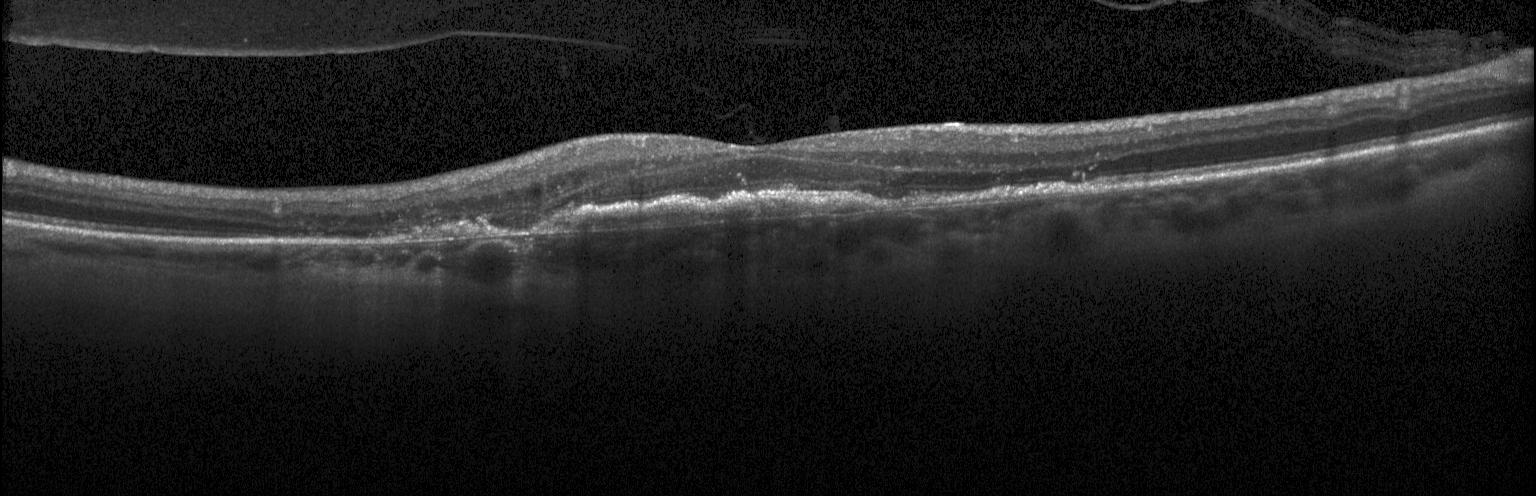 Spectral-domain OCT, optical coherence tomography scan, Heidelberg Spectralis, centered on the fovea. Choroidal neovascularization (CNV).